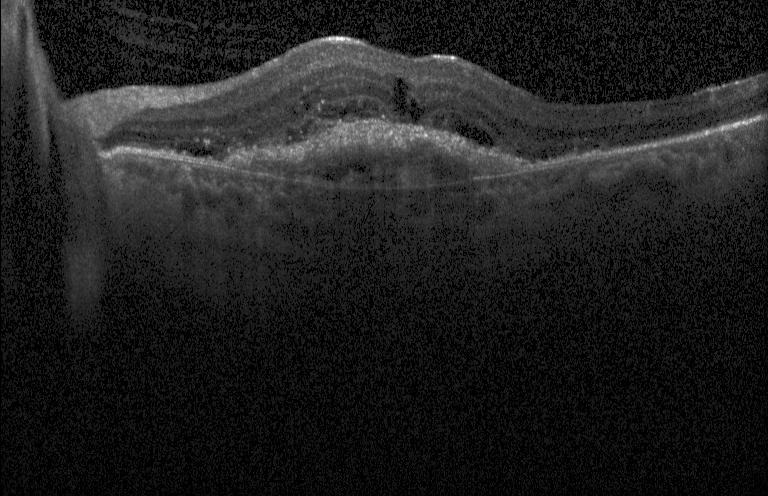 Heidelberg Spectralis OCT system. SD-OCT. Optical coherence tomography B-scan. Macular OCT: choroidal neovascularization.